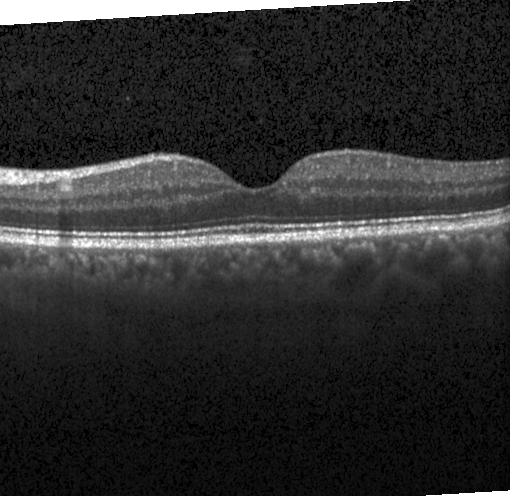

Retinal OCT cross-section showing no CNV, no DME, and no drusen.